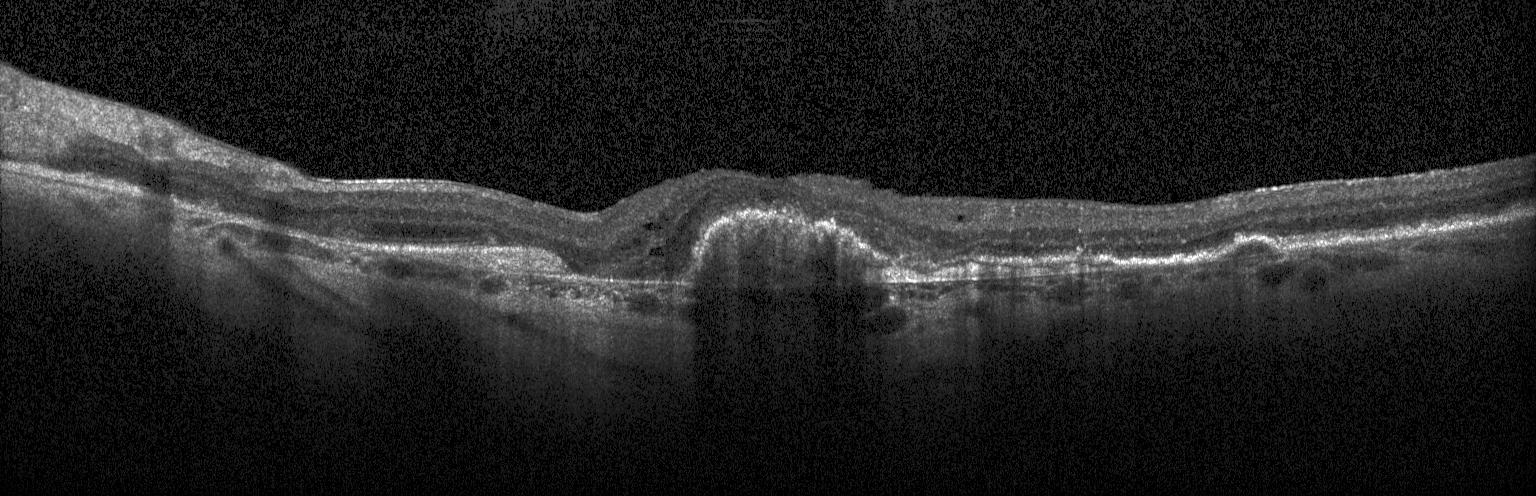
Optical coherence tomography scan
Finding: choroidal neovascularization (CNV).